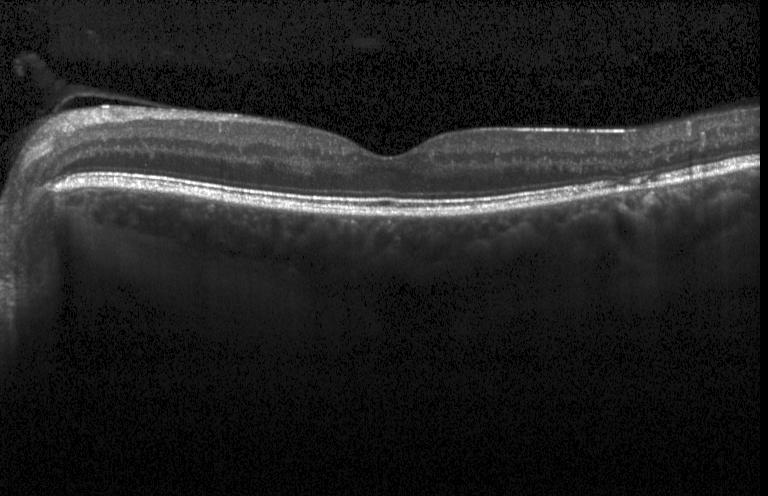

Spectral-domain OCT B-scan: no evidence of CNV, DME, or drusen.